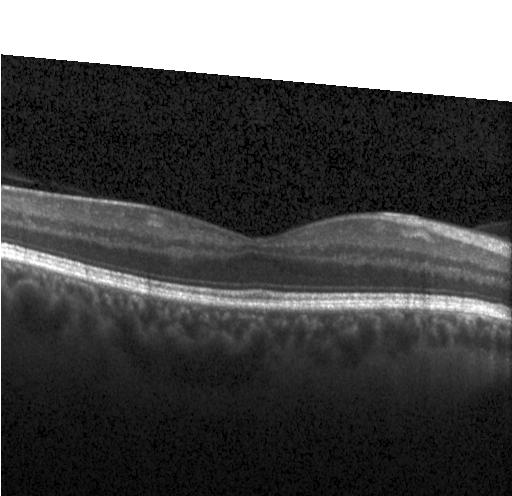
Diagnosis: no choroidal neovascularization, diabetic macular edema, or drusen.